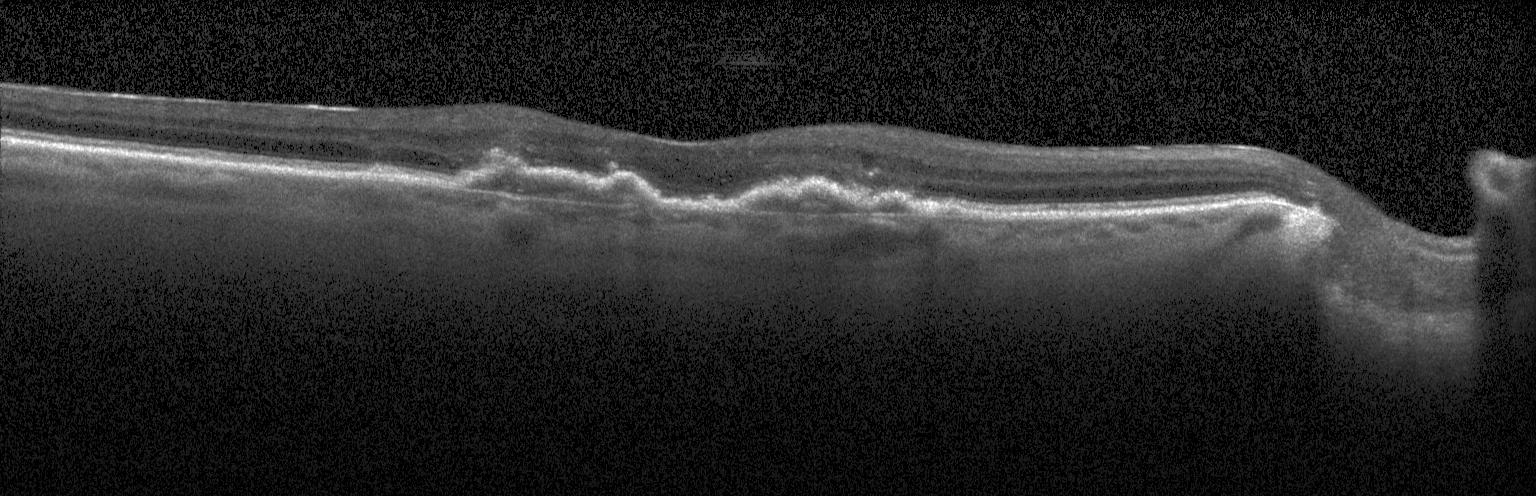 Fovea-centered. Spectral-domain optical coherence tomography. Optical coherence tomography scan. Heidelberg Spectralis
Assessment: a choroidal neovascular membrane.